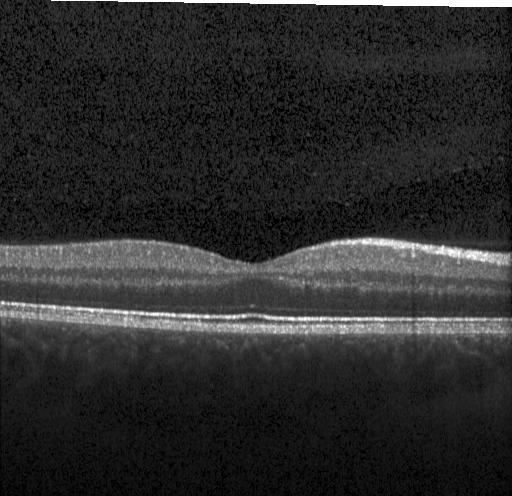 Horizontal scan through the fovea. Retinal OCT B-scan.
No CNV, no DME, and no drusen.